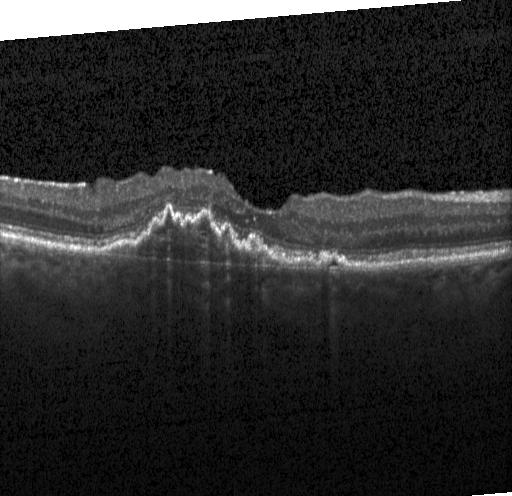
Retinal OCT cross-section.
OCT finding: choroidal neovascularization.